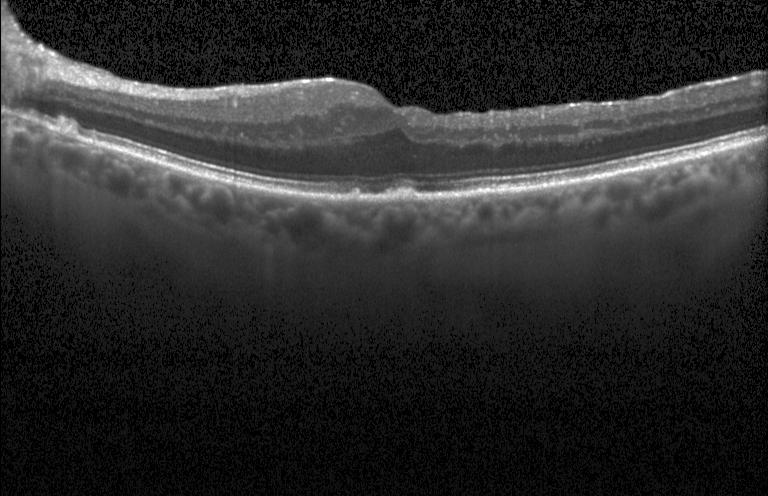 Acquired on a Heidelberg Spectralis. Through the macula. OCT B-scan. Spectral-domain optical coherence tomography. Macular OCT: drusen.